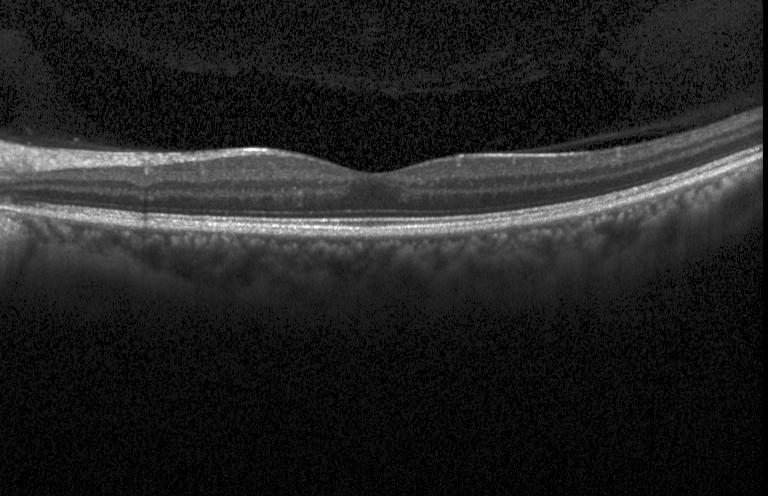 Dx: neither choroidal neovascularization, diabetic macular edema, nor drusen.